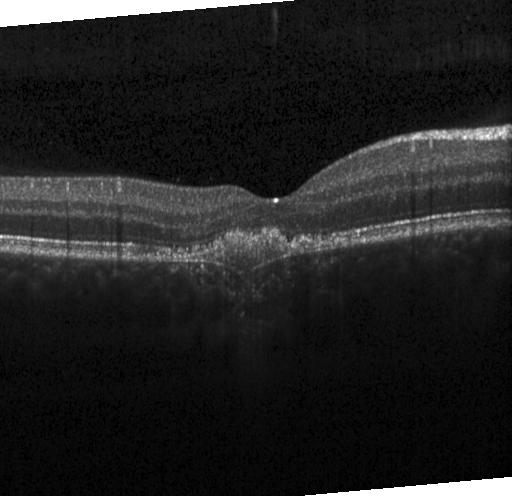
Spectral-domain optical coherence tomography. Centered on the fovea. Retinal OCT cross-section
Macular OCT: CNV.